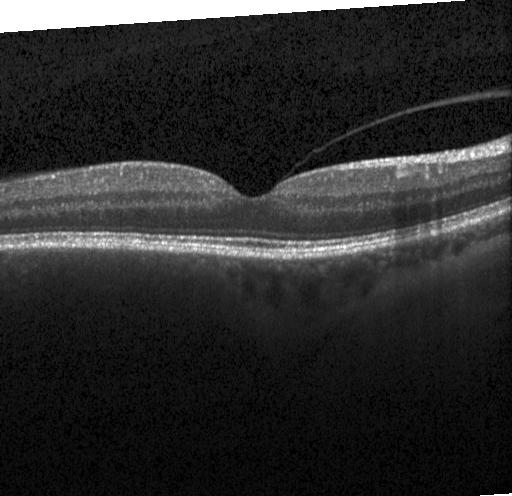

Spectral-domain OCT B-scan: no choroidal neovascularization, no diabetic macular edema, and no drusen.